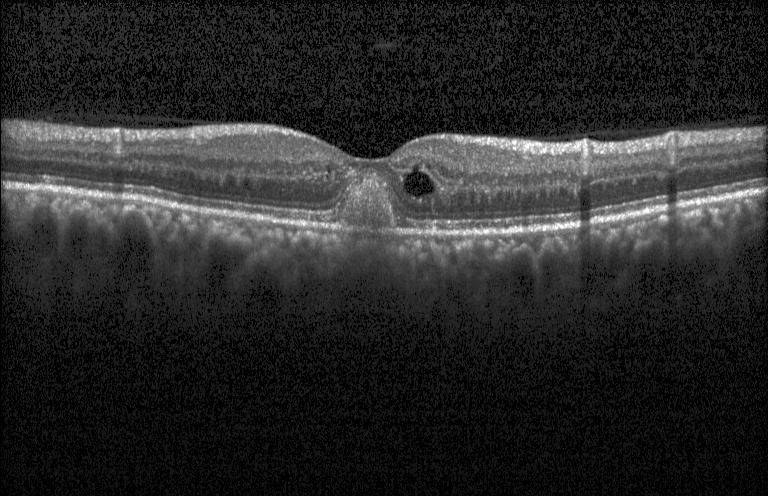
Centered on the fovea; SD-OCT; optical coherence tomography B-scan.
The scan shows a choroidal neovascular membrane.